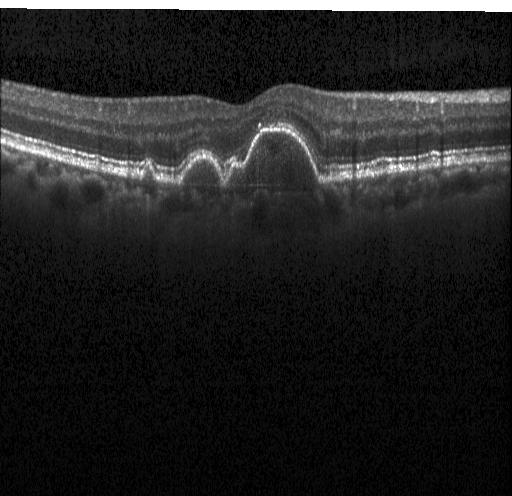 Assessment: multiple drusen.